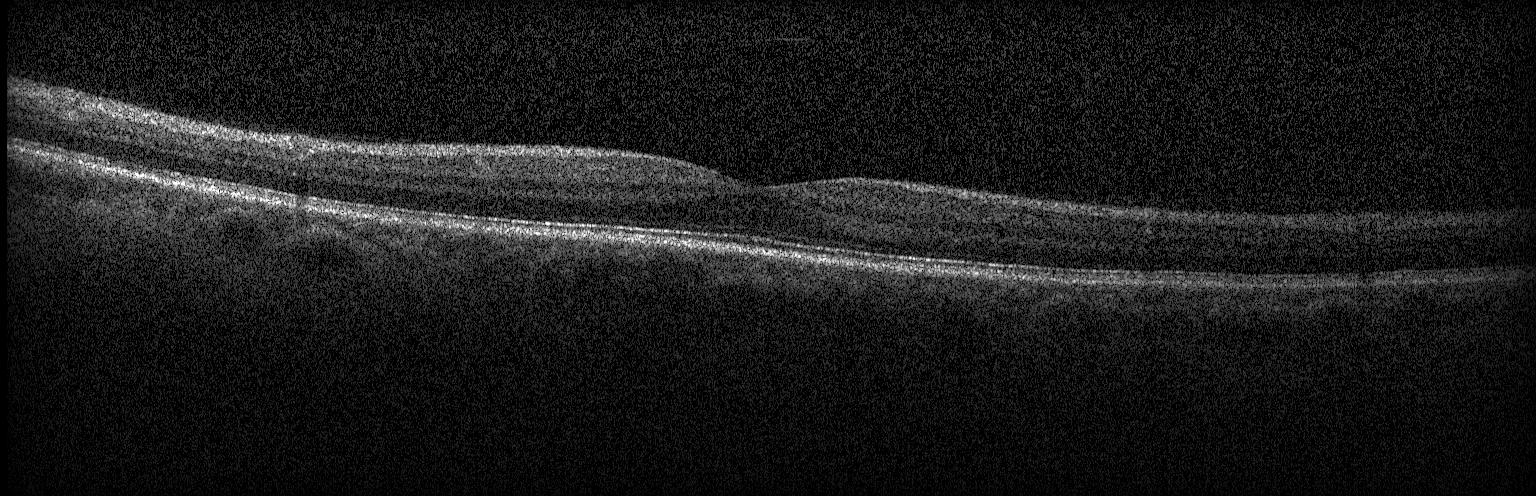
Retinal OCT cross-section
Assessment: no evidence of choroidal neovascularization, diabetic macular edema, or drusen.